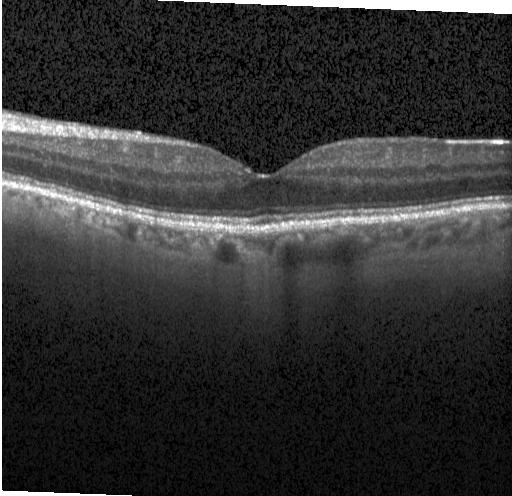
Retinal OCT cross-section; horizontal scan through the fovea; SD-OCT
The scan shows neither choroidal neovascularization, diabetic macular edema, nor drusen.